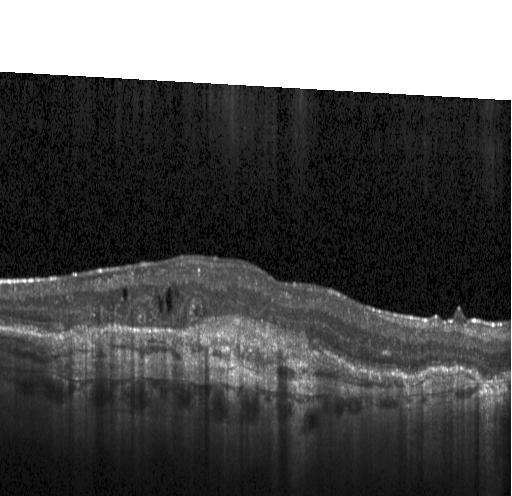 Acquired on a Heidelberg Spectralis · retinal OCT cross-section
Impression: a choroidal neovascular membrane.